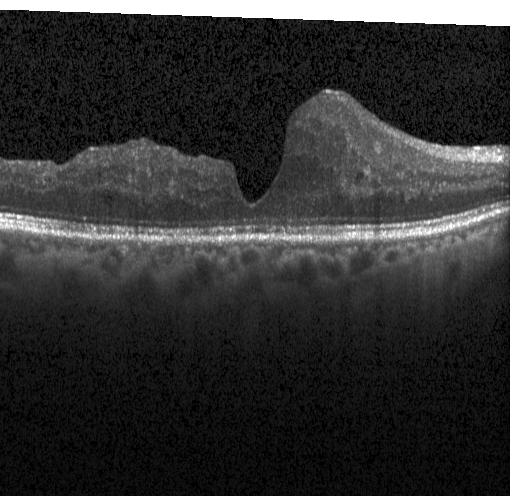

Spectral-domain optical coherence tomography; retinal OCT B-scan
Diagnosis: diabetic macular edema (DME).